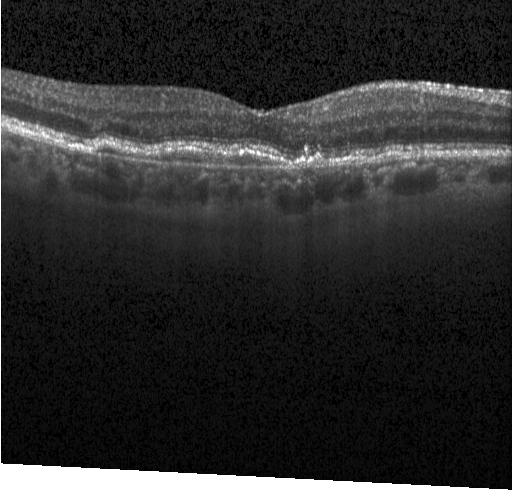 Impression: choroidal neovascularization (CNV).